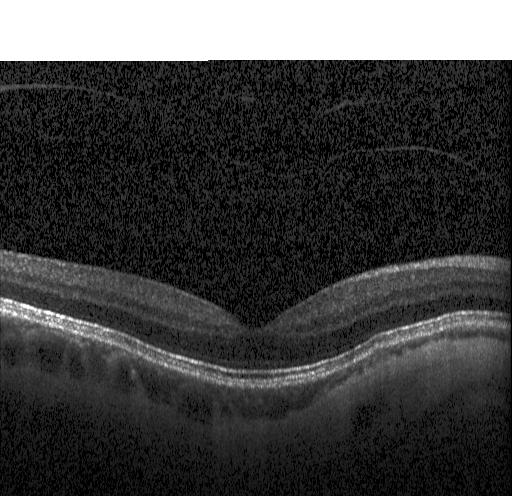
Retinal OCT cross-section
Impression: no CNV, no DME, and no drusen.